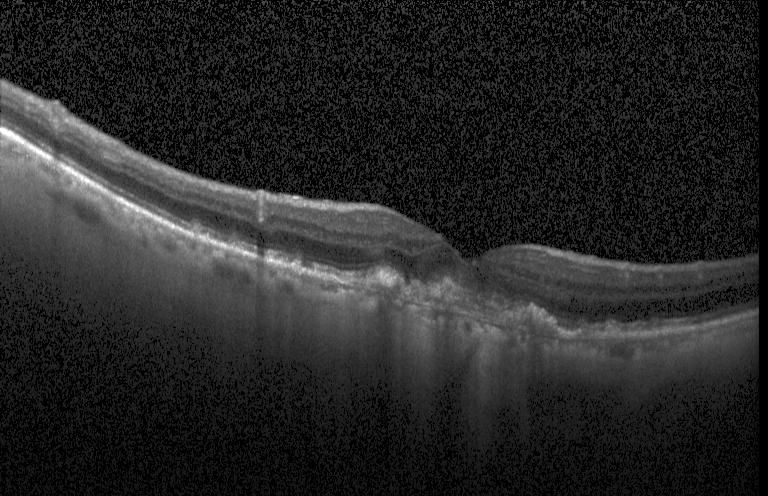

Heidelberg Spectralis, optical coherence tomography scan, horizontal scan through the fovea. Diagnosis: choroidal neovascularization (CNV).